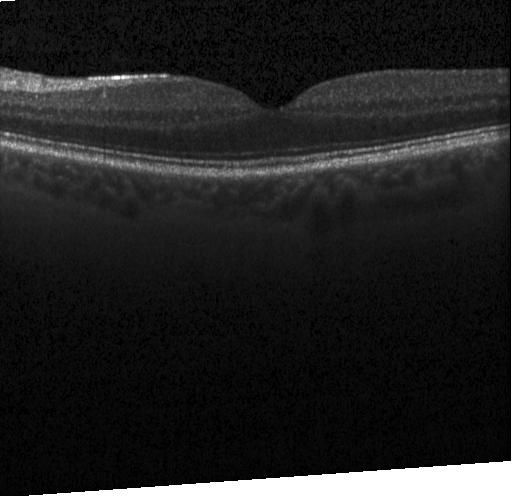

Centered on the fovea; optical coherence tomography scan; SD-OCT. This B-scan demonstrates no choroidal neovascularization, no diabetic macular edema, and no drusen.